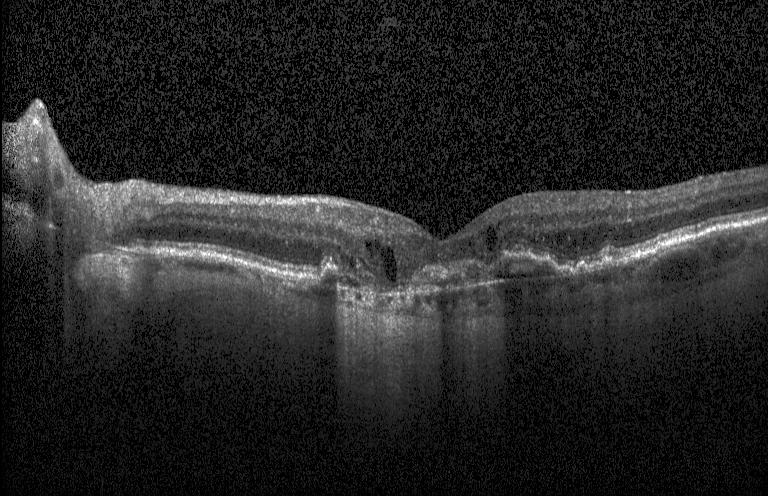

Finding: CNV.